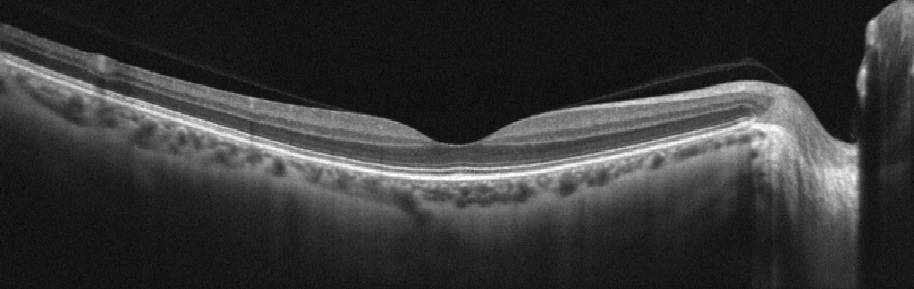

Fovea-centered. Optical coherence tomography B-scan. Optovue Avanti RTVue XR
Diagnosis: no AMD, DME, ERM, RAO, RVO, or VID.